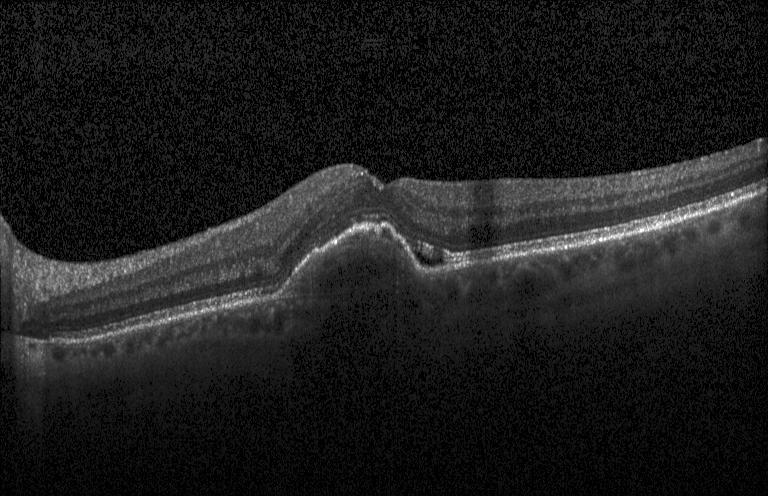 Finding: a choroidal neovascular membrane.